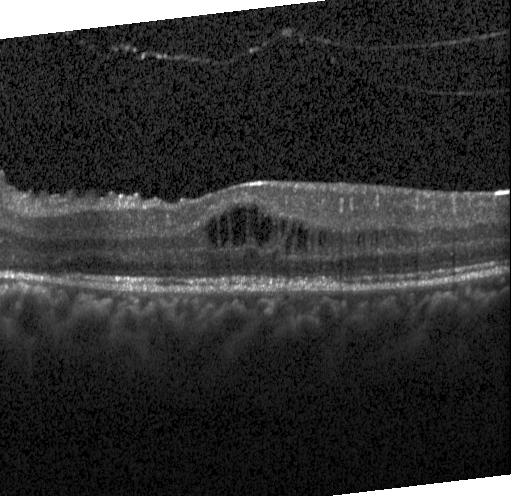 Fovea-centered. Heidelberg Spectralis OCT system. SD-OCT. OCT B-scan
Finding: DME.